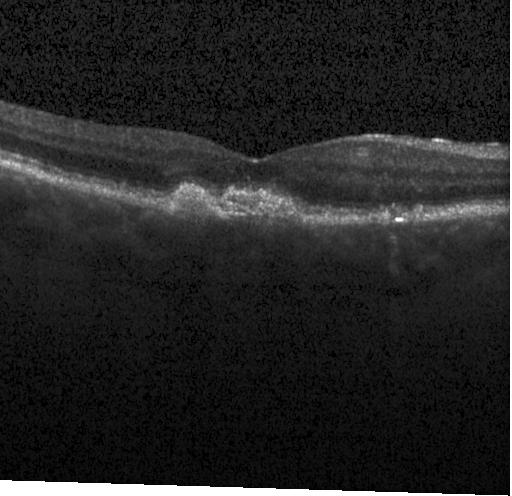
Spectral-domain OCT B-scan: choroidal neovascularization (CNV).